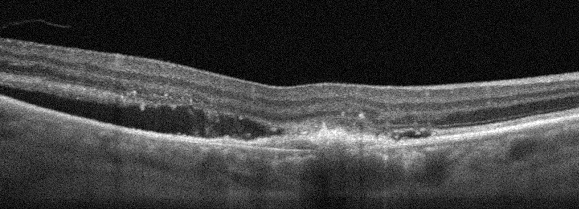
Right eye. Retinal OCT B-scan
Dx: age-related macular degeneration (AMD).